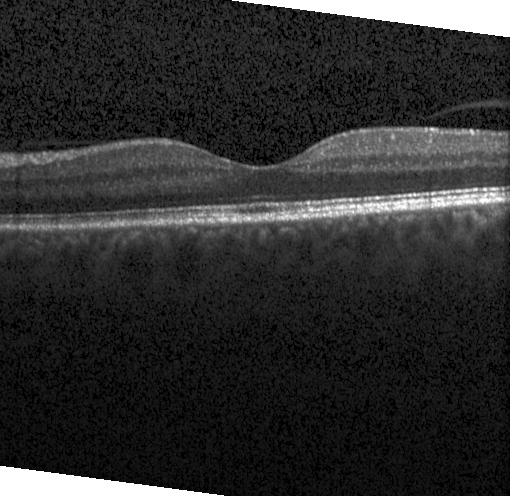

The scan shows no evidence of choroidal neovascularization, diabetic macular edema, or drusen.